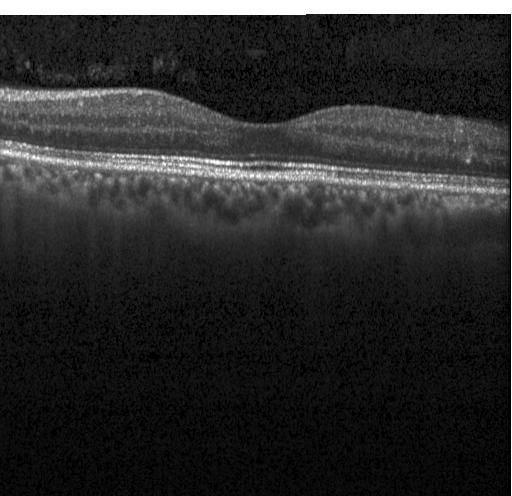 The scan shows neither CNV, DME, nor drusen.